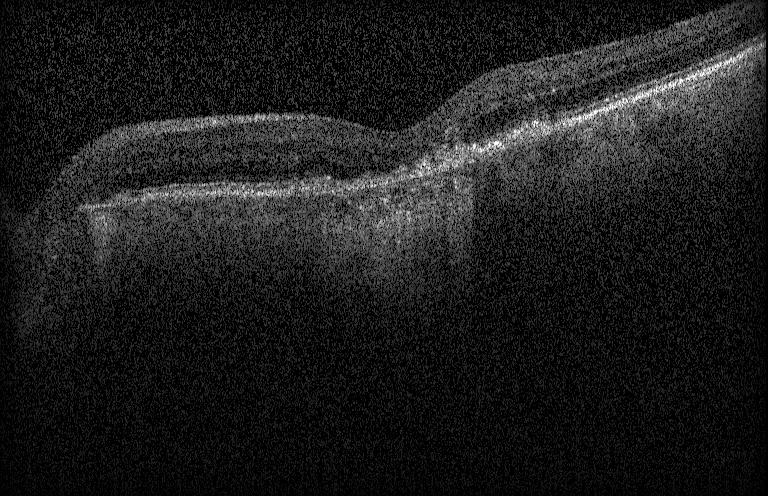
Acquired on a Heidelberg Spectralis, retinal OCT B-scan.
Macular OCT: a choroidal neovascular membrane.